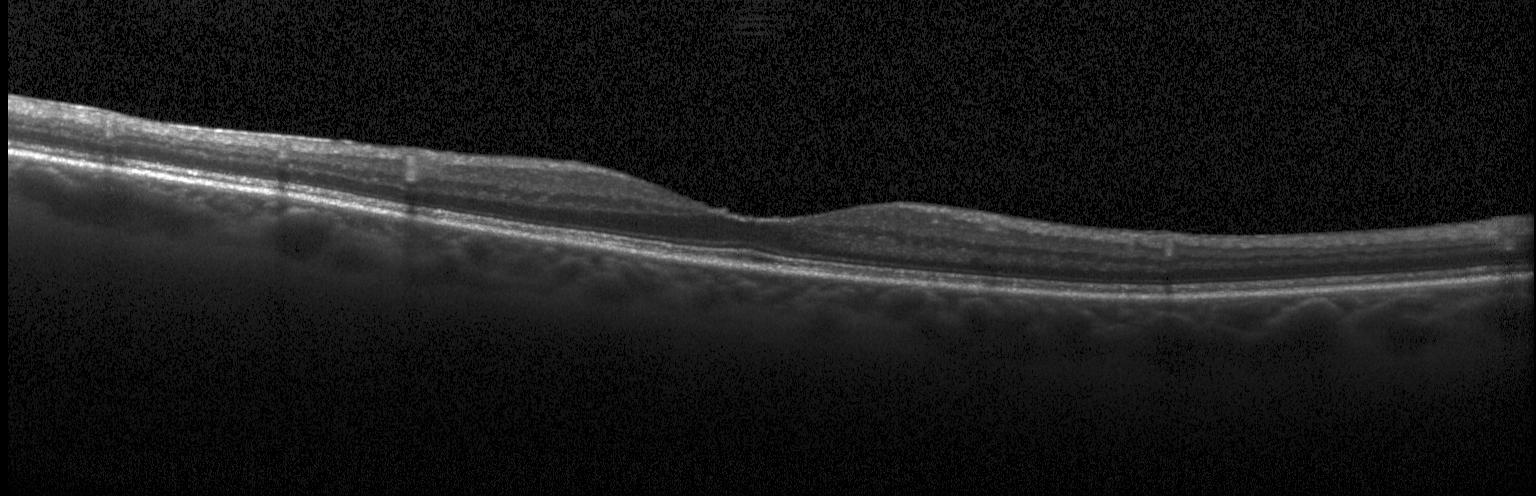
Optical coherence tomography scan. Assessment: no choroidal neovascularization, diabetic macular edema, or drusen.